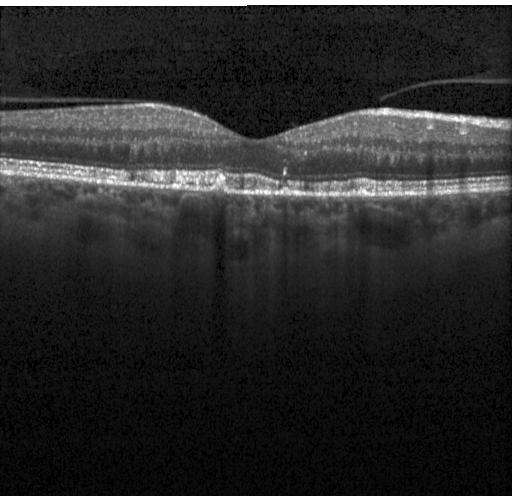
Impression: drusen.